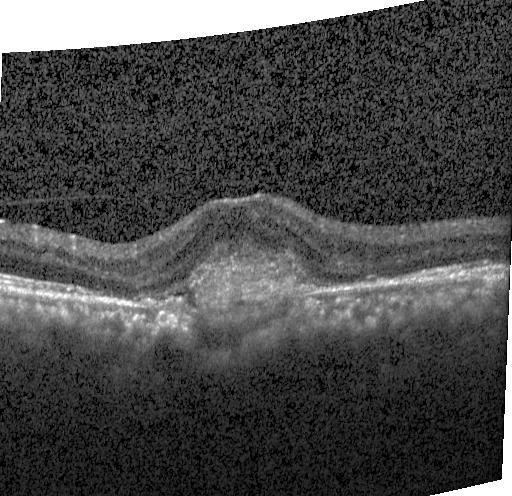 OCT B-scan — Assessment: CNV.